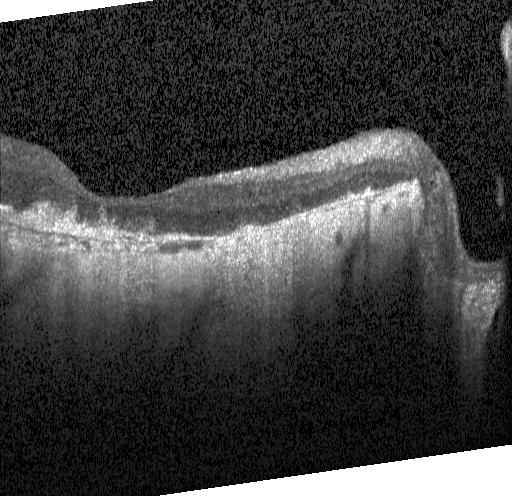 OCT line scan · instrument: Heidelberg Spectralis — The scan shows a choroidal neovascular membrane.